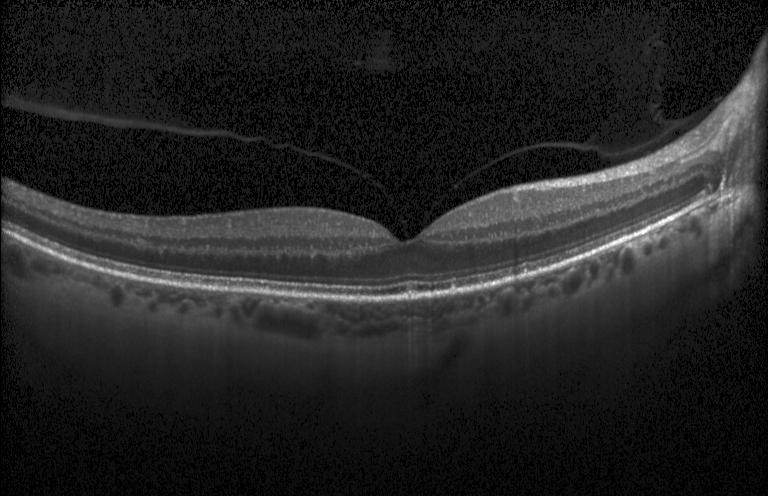
Through the macula. Spectral-domain optical coherence tomography. Retinal OCT cross-section.
This B-scan demonstrates drusen.